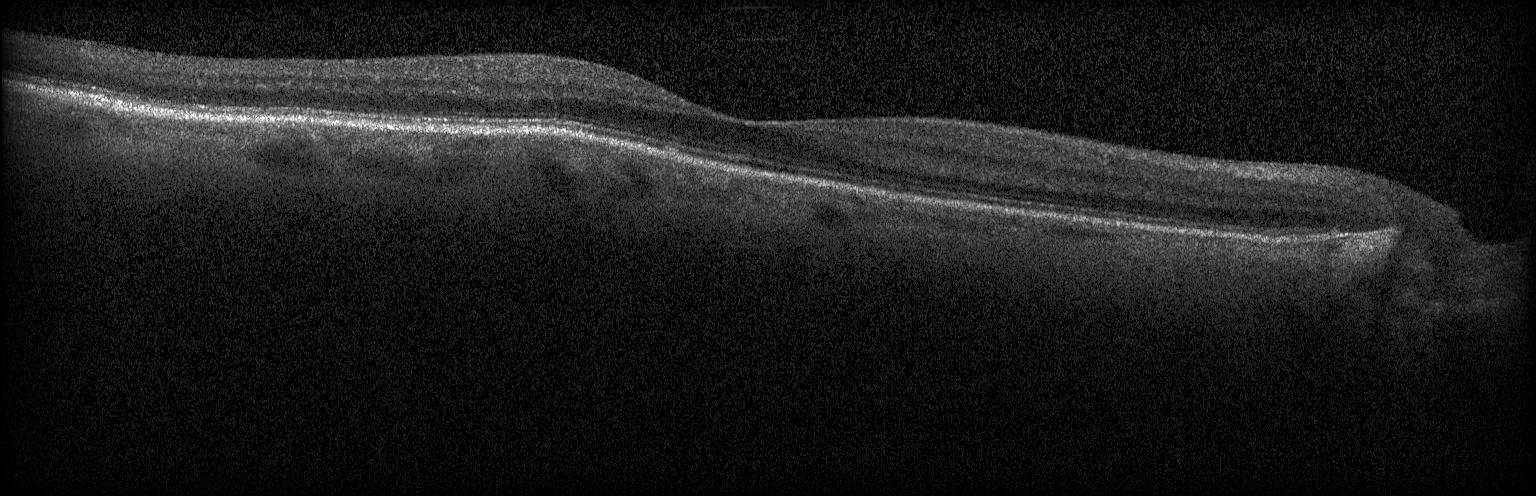 Macular OCT demonstrating no evidence of choroidal neovascularization, diabetic macular edema, or drusen.